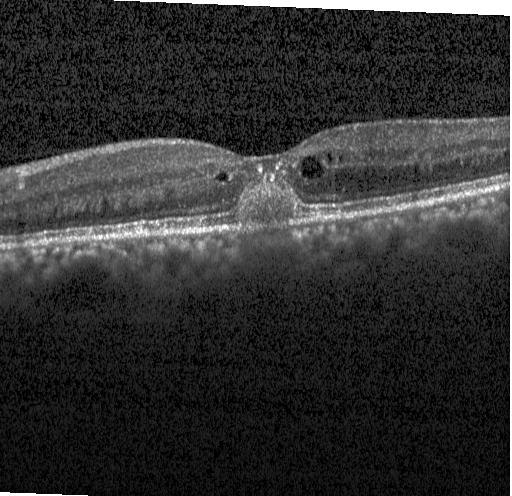
OCT line scan; through the macula
Finding: a choroidal neovascular membrane.